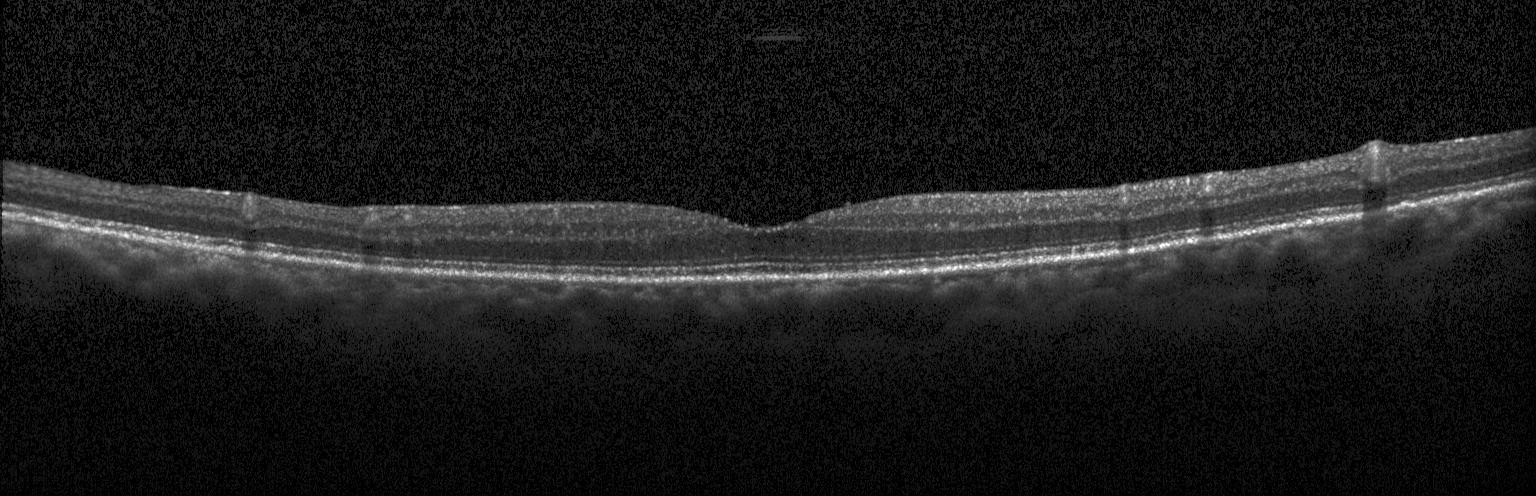
Neither choroidal neovascularization, diabetic macular edema, nor drusen.